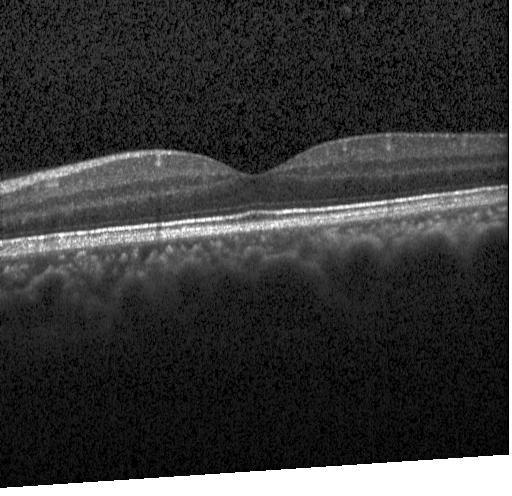
Diagnosis: no choroidal neovascularization, no diabetic macular edema, and no drusen.